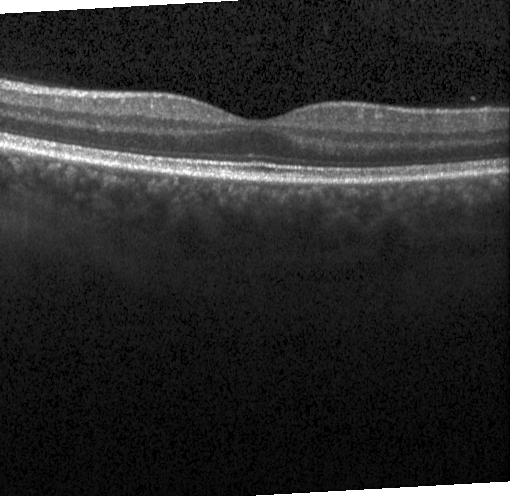 Optical coherence tomography B-scan.
Finding: no CNV, no DME, and no drusen.